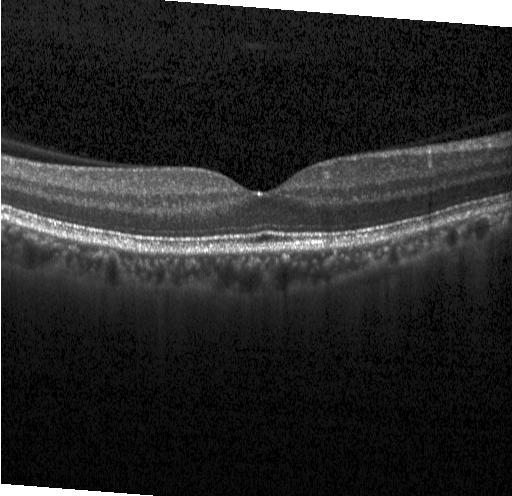 This B-scan demonstrates no choroidal neovascularization, no diabetic macular edema, and no drusen.